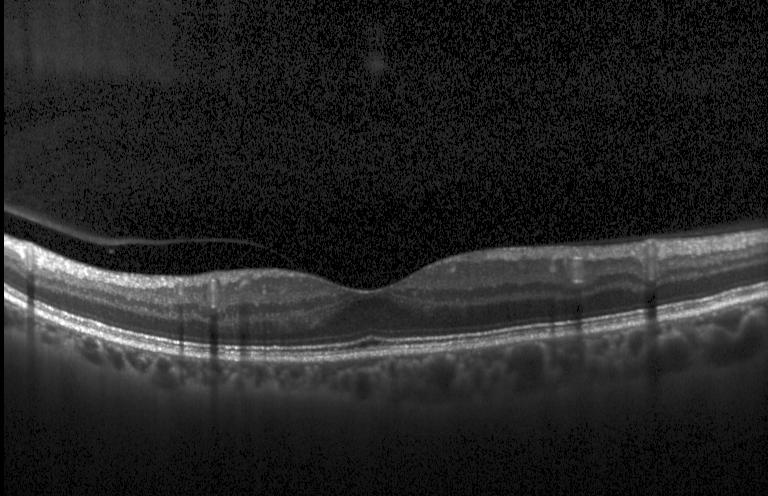 Optical coherence tomography B-scan · Heidelberg Spectralis OCT system · centered on the fovea · spectral-domain optical coherence tomography — Assessment: no evidence of choroidal neovascularization, diabetic macular edema, or drusen.